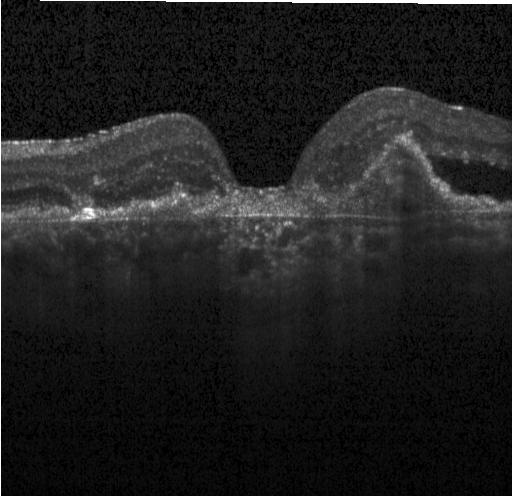 A choroidal neovascular membrane.